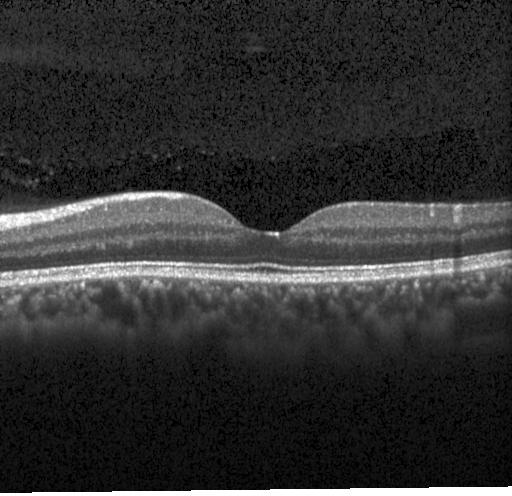
Retinal OCT B-scan. Assessment: no choroidal neovascularization, diabetic macular edema, or drusen.